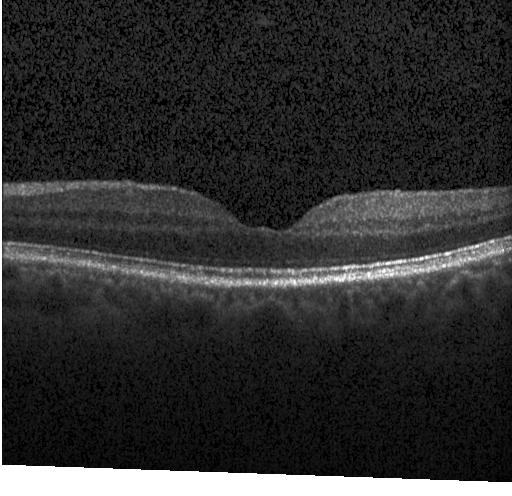
OCT finding: no choroidal neovascularization, no diabetic macular edema, and no drusen.